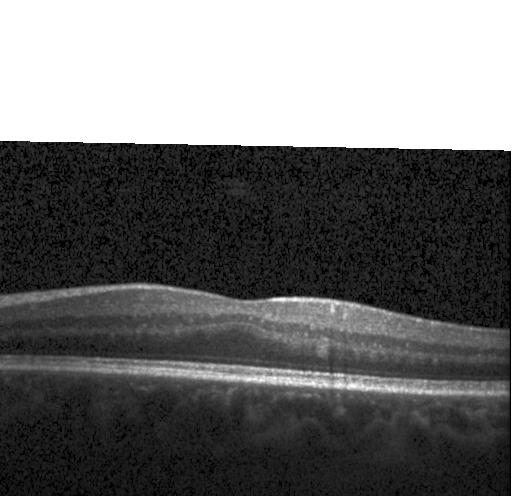

Impression: no CNV, DME, or drusen.